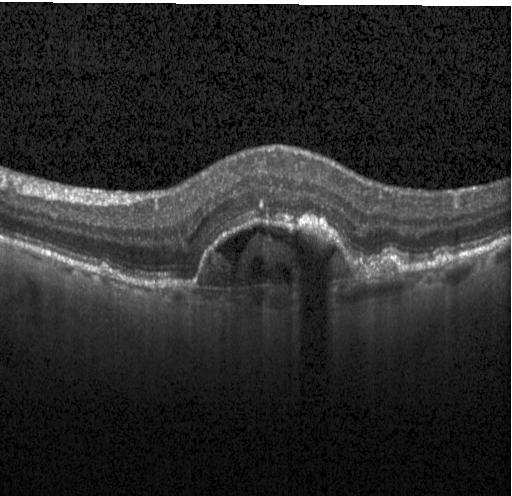

Instrument: Heidelberg Spectralis; OCT B-scan; centered on the fovea.
Dx: CNV.